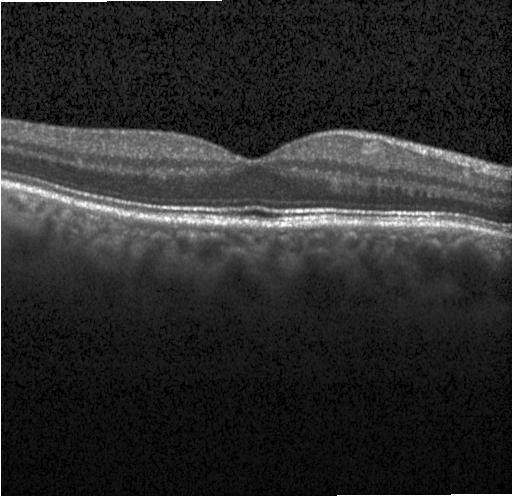 Spectral-domain optical coherence tomography. Through the macula. Optical coherence tomography scan — This B-scan demonstrates no choroidal neovascularization, diabetic macular edema, or drusen.